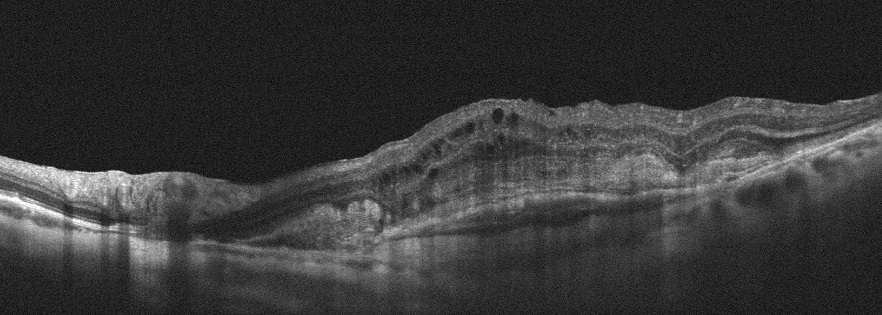 Retinal OCT B-scan. AMD.